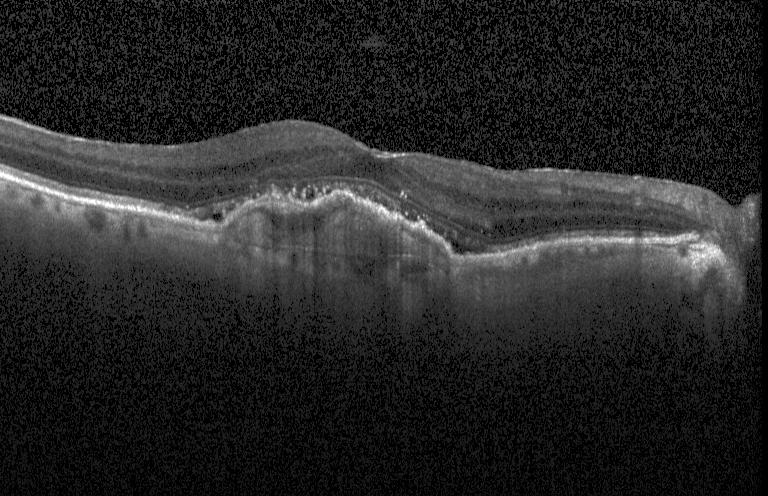 Optical coherence tomography B-scan — Assessment: choroidal neovascularization (CNV).